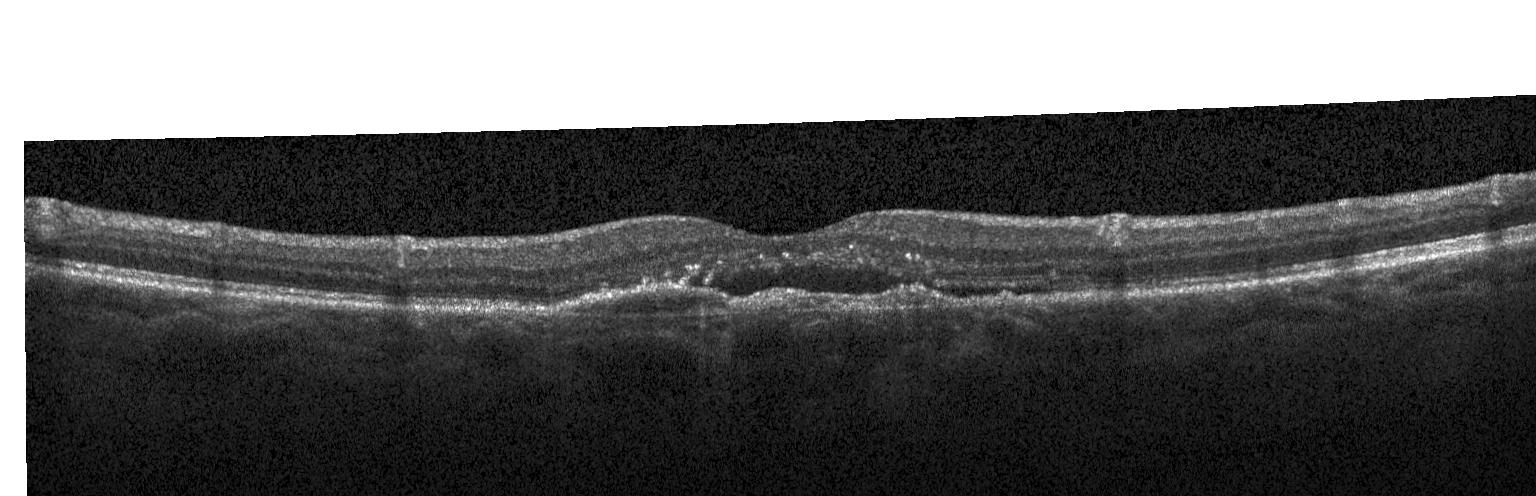 Heidelberg Spectralis · OCT B-scan
This B-scan demonstrates a choroidal neovascular membrane.